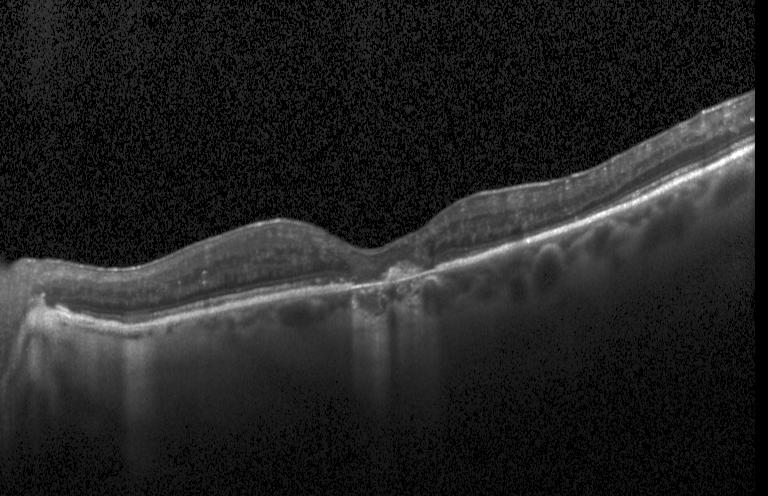
Fovea-centered, optical coherence tomography scan, acquired on a Heidelberg Spectralis. Diagnosis: choroidal neovascularization.